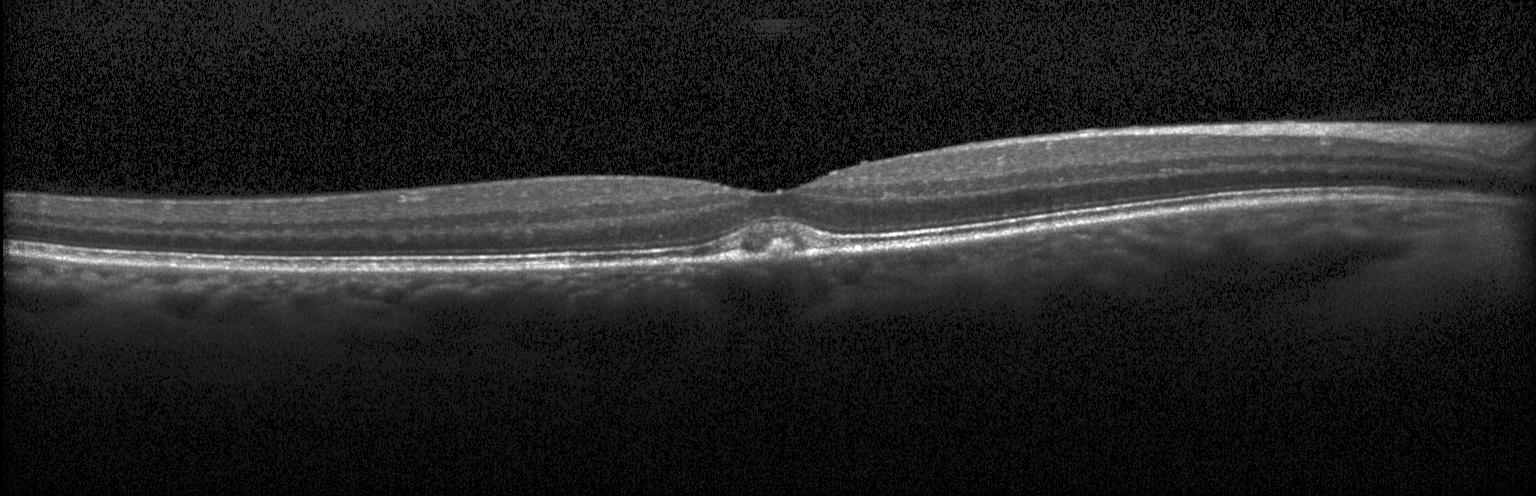

Acquired on a Heidelberg Spectralis, macular scan, spectral-domain optical coherence tomography, OCT B-scan.
This B-scan demonstrates choroidal neovascularization (CNV).